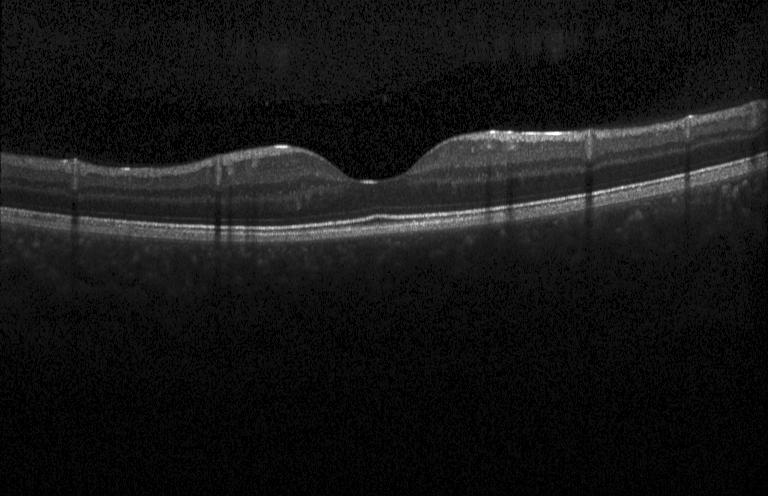

OCT B-scan showing neither CNV, DME, nor drusen.